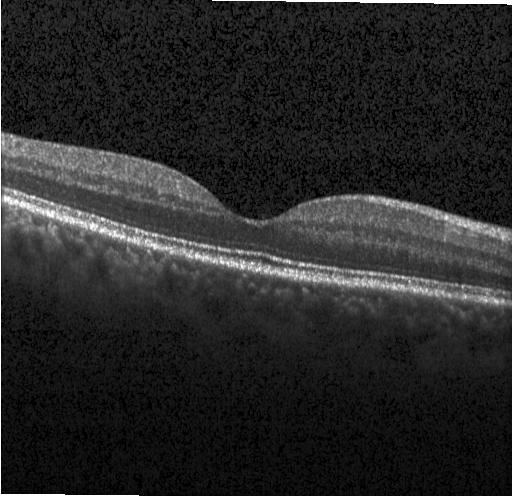 OCT scan showing no choroidal neovascularization, no diabetic macular edema, and no drusen.